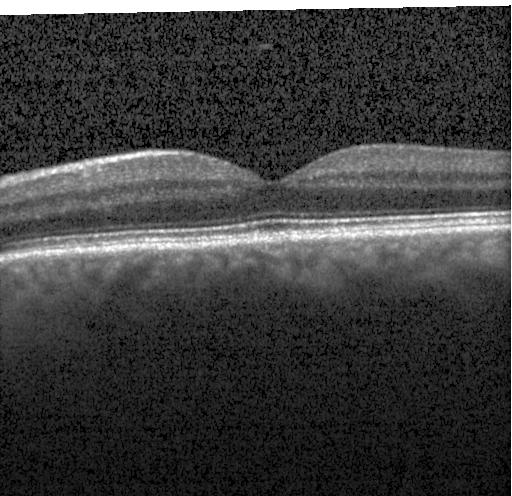

Through the macula; OCT line scan
Macular OCT: neither choroidal neovascularization, diabetic macular edema, nor drusen.